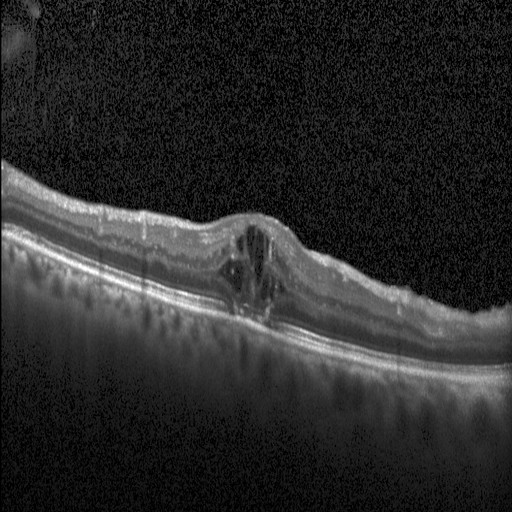
Spectral-domain OCT · horizontal scan through the fovea · instrument: Heidelberg Spectralis · OCT line scan — Finding: DME.